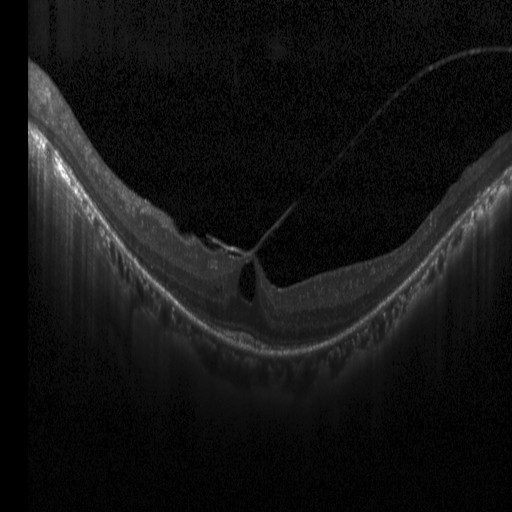
Retinal OCT cross-section showing diabetic macular edema (DME).